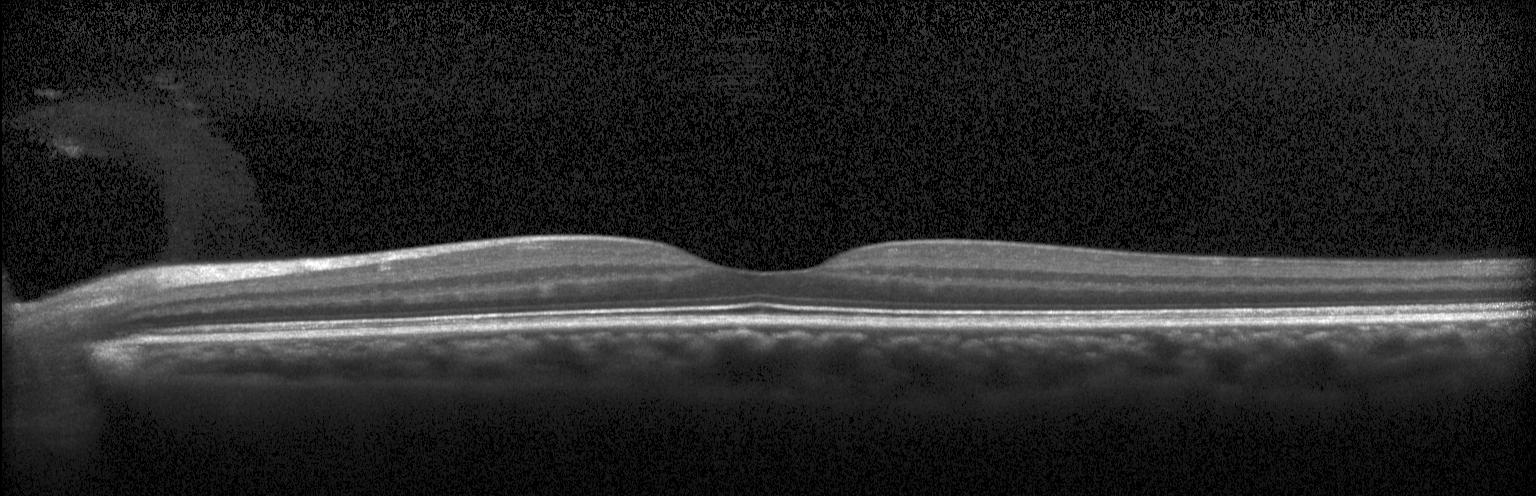 OCT B-scan. Centered on the fovea. Spectral-domain OCT. Acquired on a Heidelberg Spectralis.
The scan shows no choroidal neovascularization, no diabetic macular edema, and no drusen.